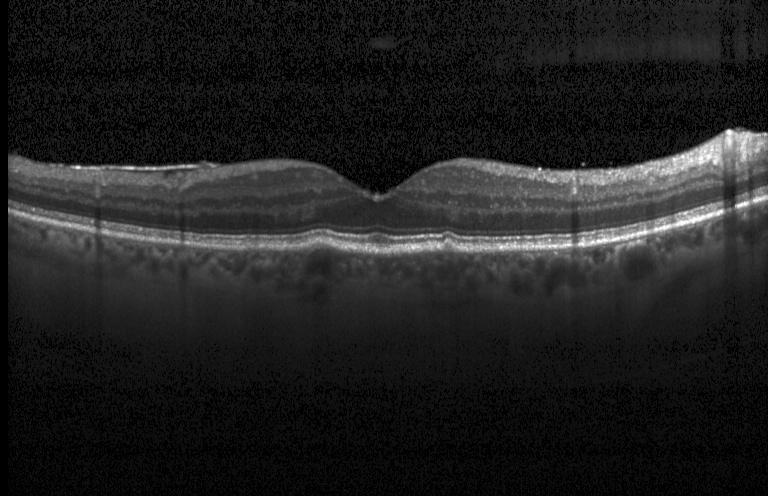 Fovea-centered; retinal OCT cross-section; SD-OCT. Impression: drusen.